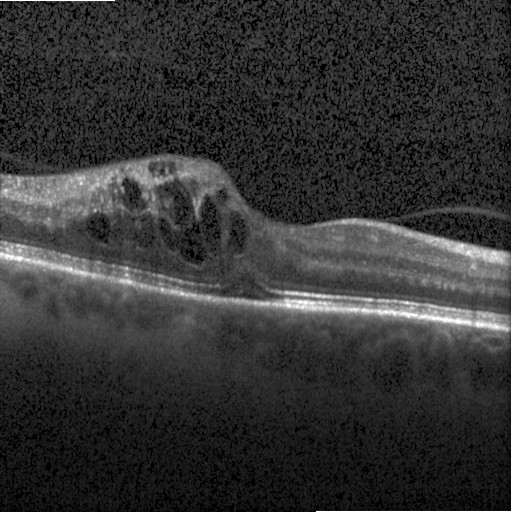
Spectral-domain optical coherence tomography, optical coherence tomography B-scan, instrument: Heidelberg Spectralis — Macular OCT: diabetic macular edema.